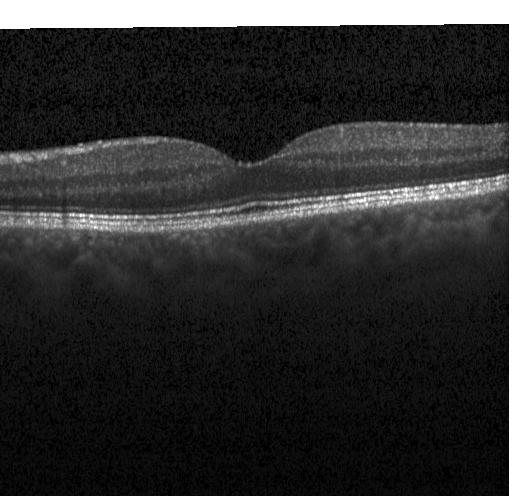 SD-OCT · horizontal scan through the fovea · optical coherence tomography scan — No choroidal neovascularization, no diabetic macular edema, and no drusen.